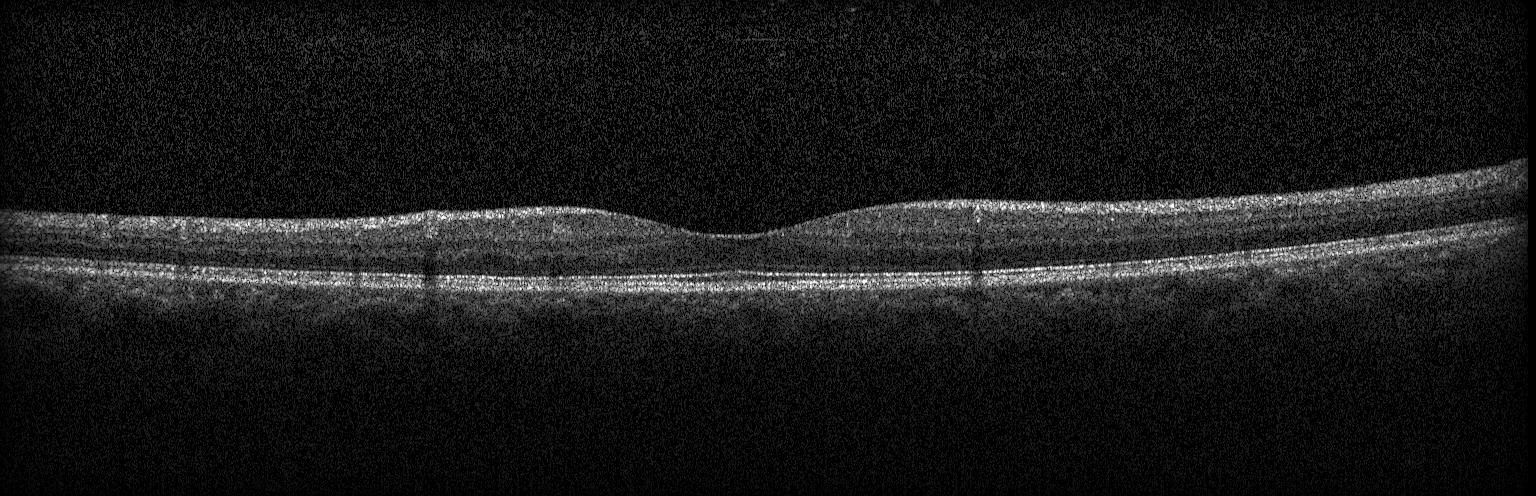
Heidelberg Spectralis; optical coherence tomography scan; spectral-domain optical coherence tomography. Macular OCT: neither CNV, DME, nor drusen.